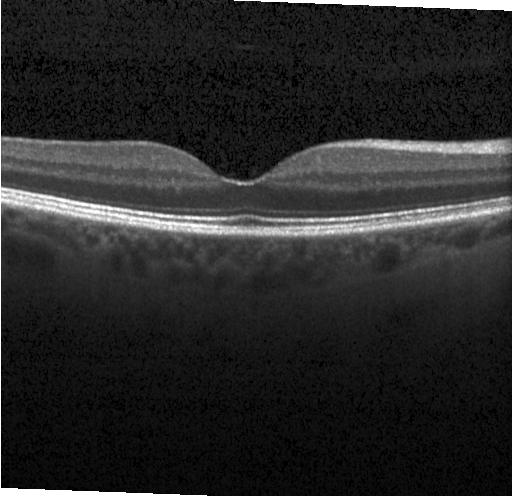
Retinal OCT cross-section; spectral-domain OCT; centered on the fovea. Impression: neither CNV, DME, nor drusen.